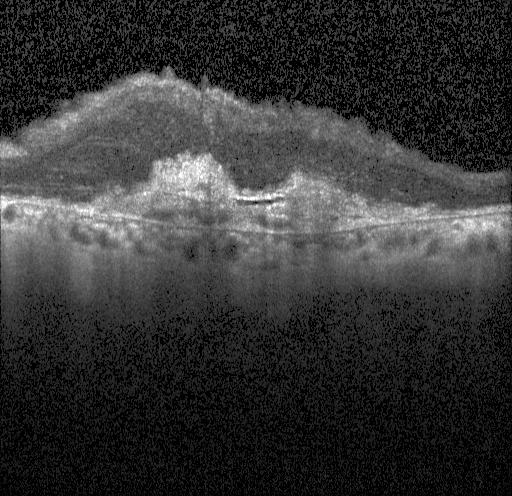 Optical coherence tomography B-scan, SD-OCT, Heidelberg Spectralis, macular scan — Finding: a choroidal neovascular membrane.